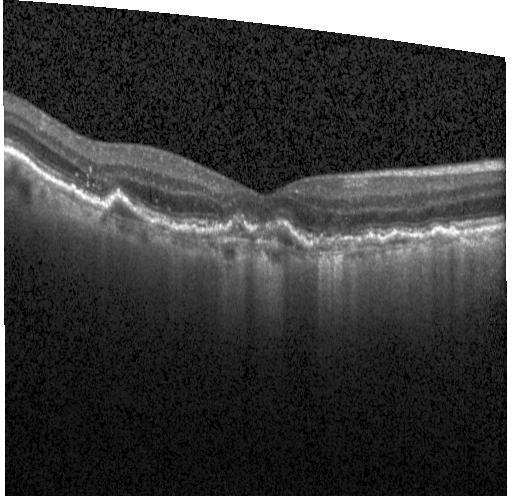 OCT B-scan — The scan shows choroidal neovascularization (CNV).